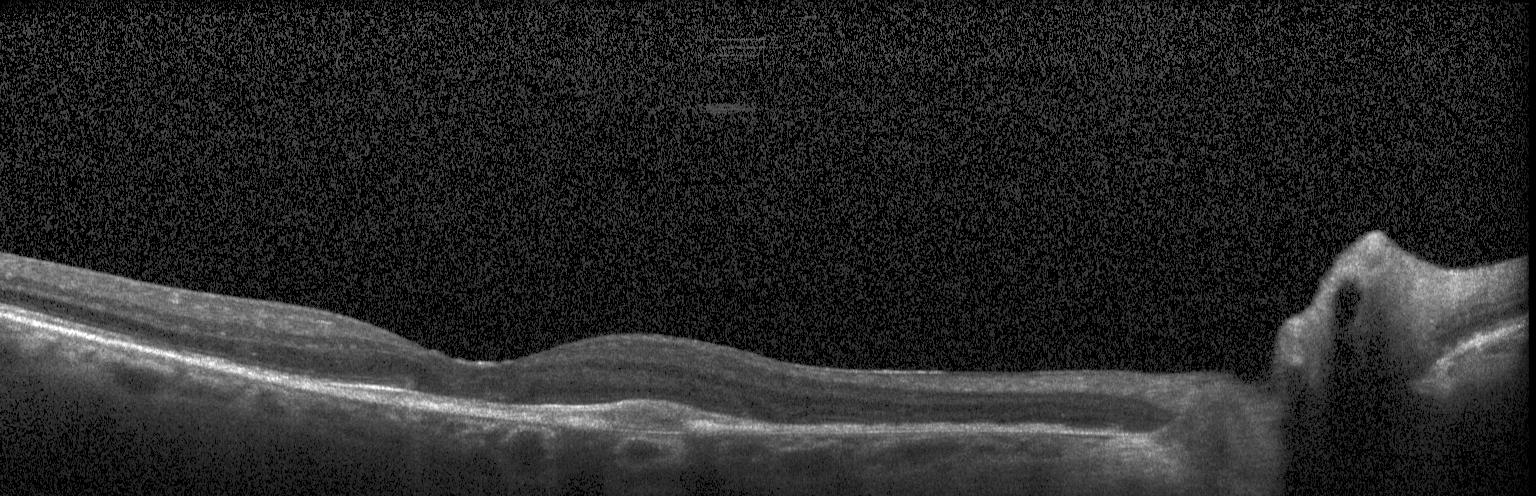

Centered on the fovea. Retinal OCT cross-section. Instrument: Heidelberg Spectralis. Spectral-domain optical coherence tomography — Macular OCT: a choroidal neovascular membrane.